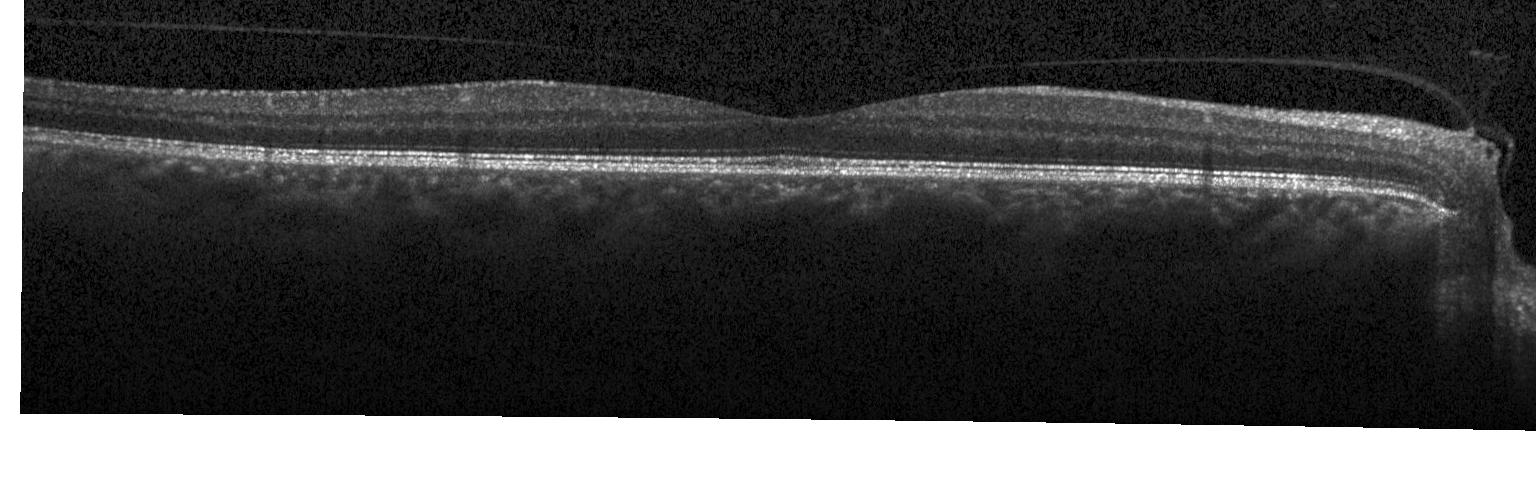
Macular OCT: no CNV, no DME, and no drusen.